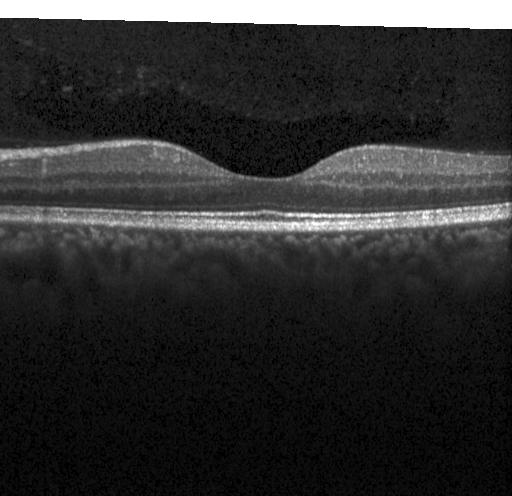

Macular scan. Heidelberg Spectralis OCT system. Optical coherence tomography scan. SD-OCT. OCT finding: neither CNV, DME, nor drusen.